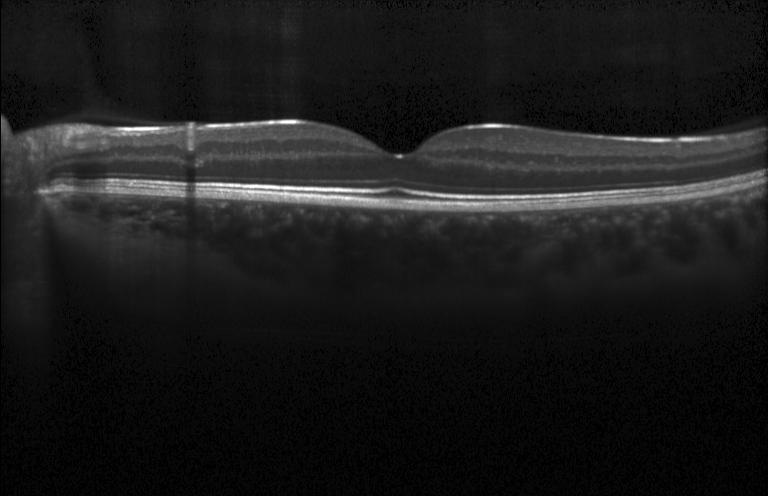
Impression: no choroidal neovascularization, diabetic macular edema, or drusen.